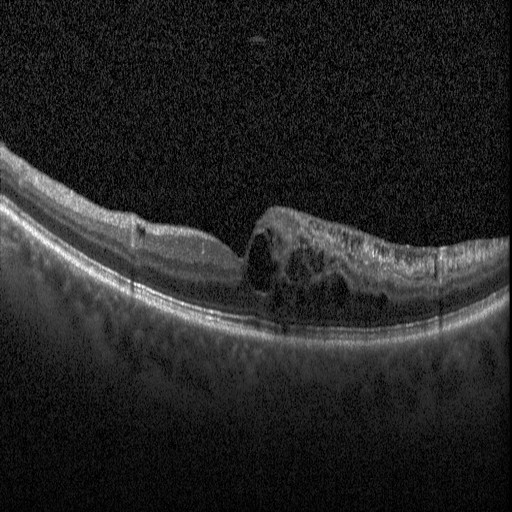

OCT B-scan showing DME.